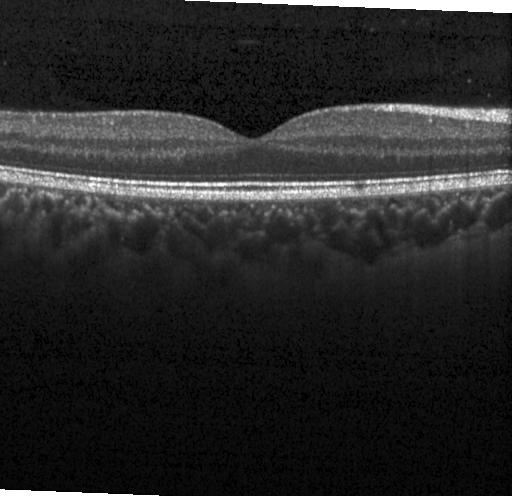 OCT B-scan.
Diagnosis: no evidence of CNV, DME, or drusen.